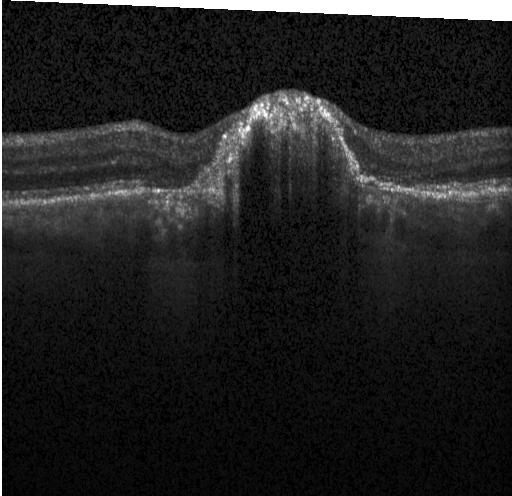

Diagnosis: CNV.